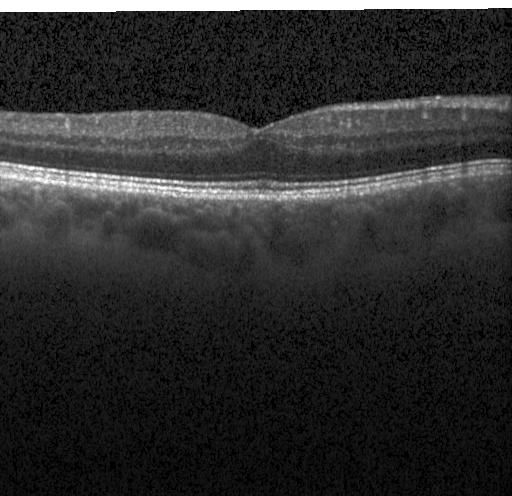

Finding: no evidence of CNV, DME, or drusen.